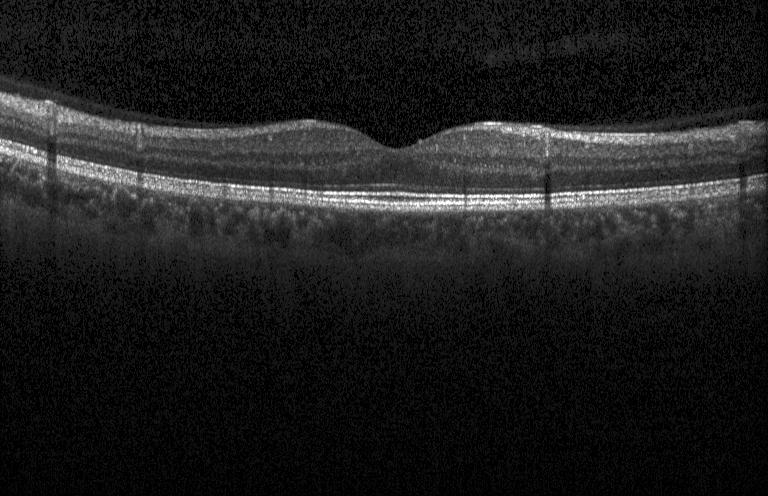

Diagnosis: neither choroidal neovascularization, diabetic macular edema, nor drusen.